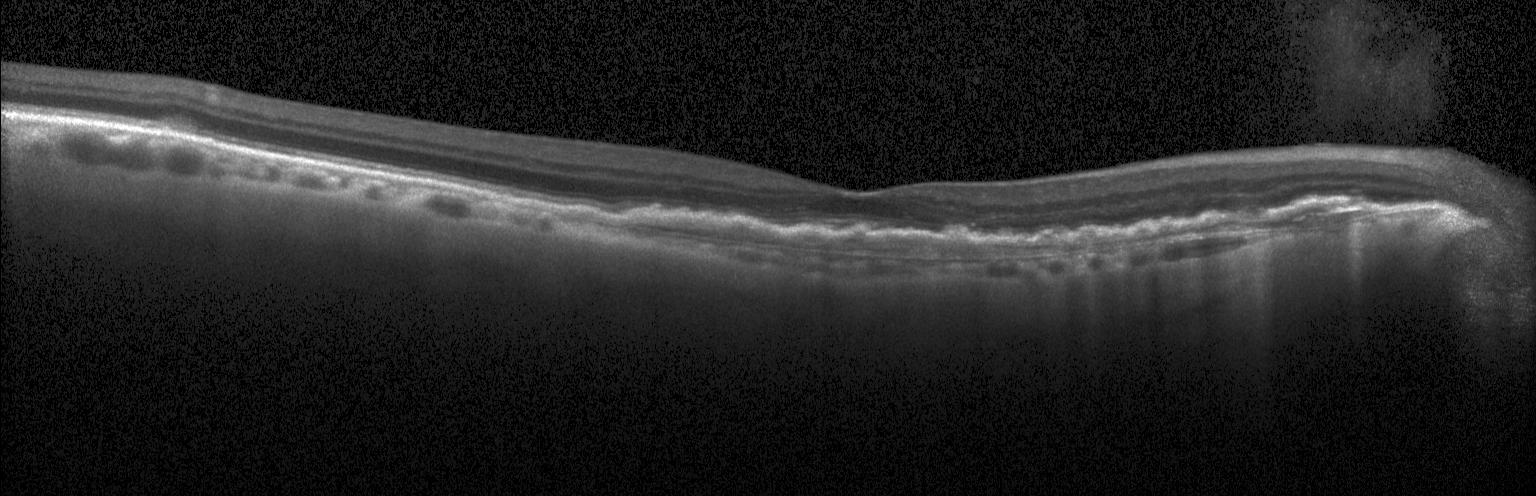 Optical coherence tomography B-scan, macular scan, instrument: Heidelberg Spectralis, spectral-domain OCT — Assessment: a choroidal neovascular membrane.